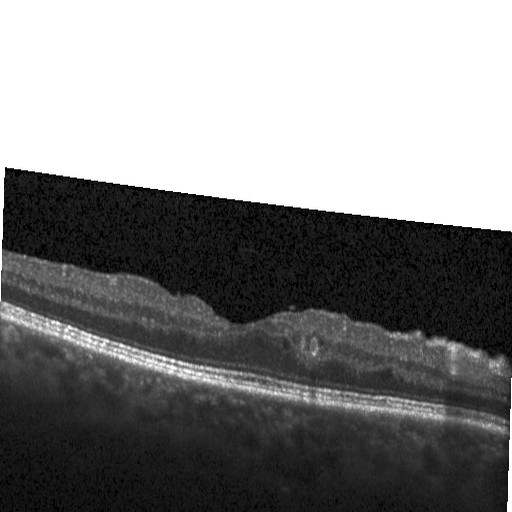 Impression: DME.